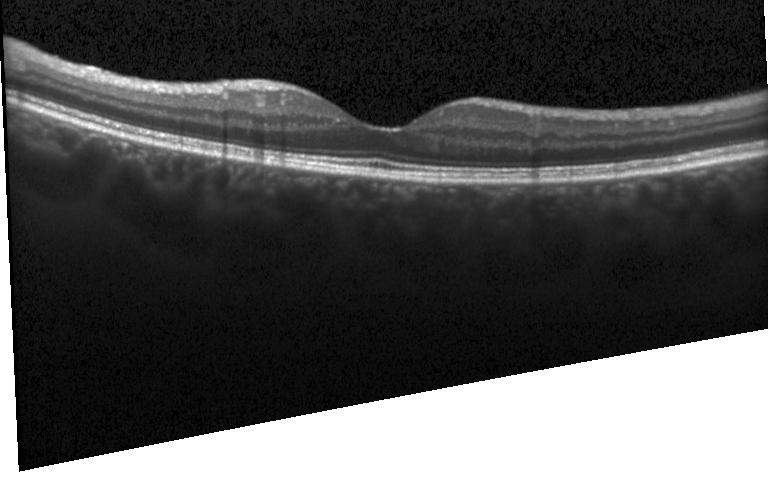

OCT B-scan. Finding: neither choroidal neovascularization, diabetic macular edema, nor drusen.